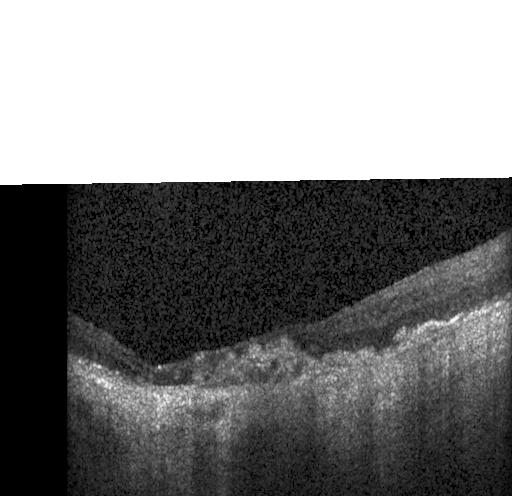

Choroidal neovascularization.